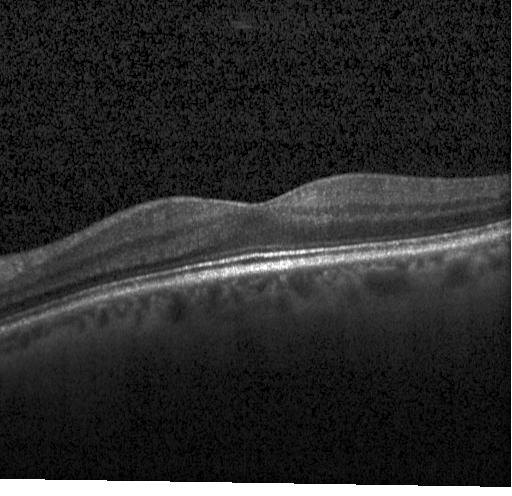 Optical coherence tomography scan; acquired on a Heidelberg Spectralis; horizontal scan through the fovea. Diagnosis: no choroidal neovascularization, diabetic macular edema, or drusen.